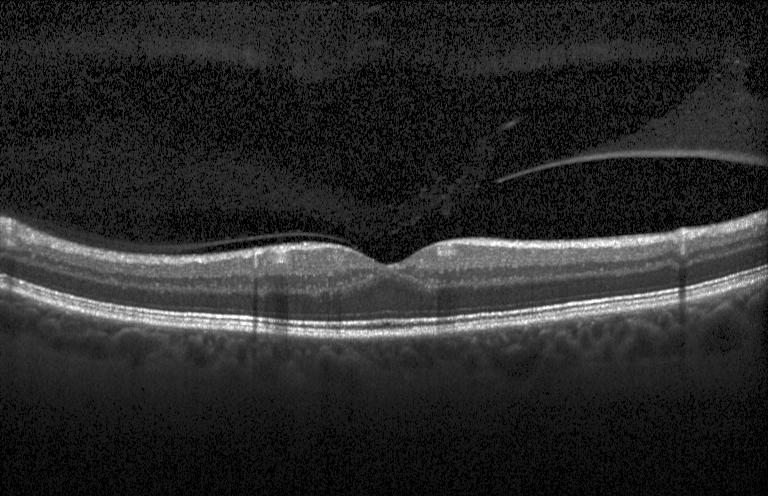 OCT scan showing no evidence of choroidal neovascularization, diabetic macular edema, or drusen.